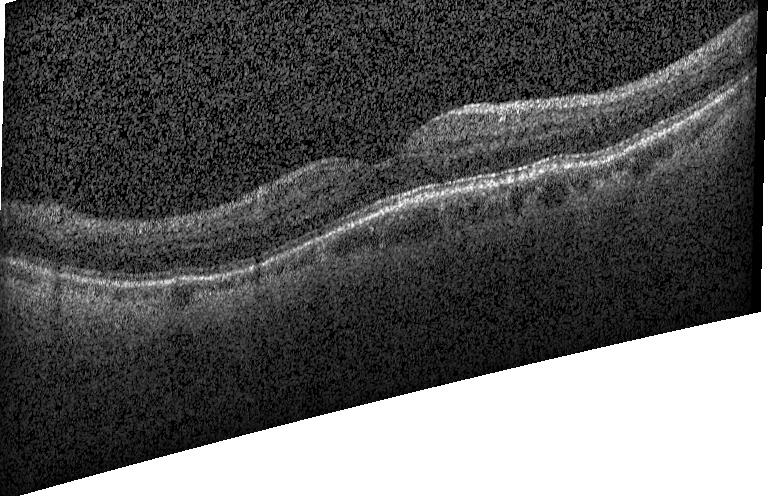

Retinal OCT B-scan; SD-OCT; horizontal scan through the fovea. Macular OCT: no CNV, DME, or drusen.